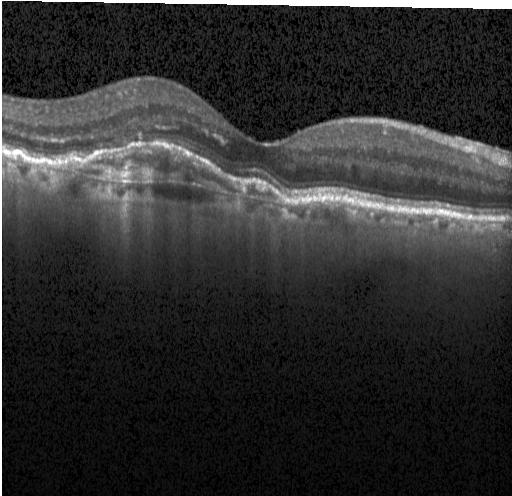
A choroidal neovascular membrane.